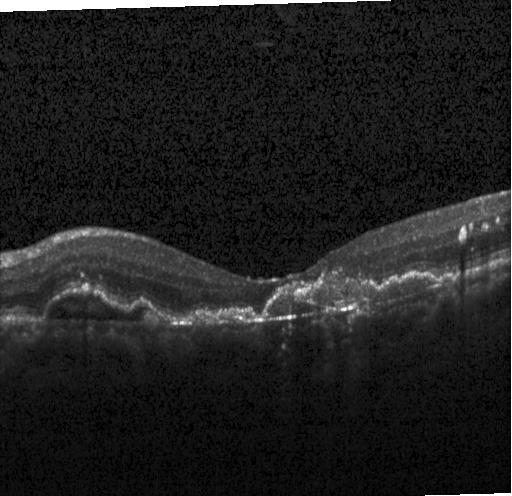

Optical coherence tomography scan.
This B-scan demonstrates a choroidal neovascular membrane.